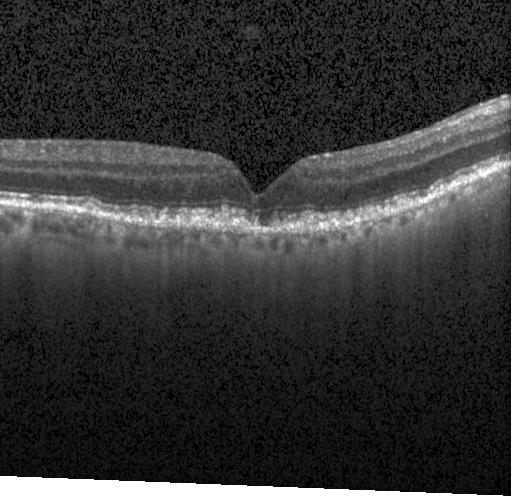

OCT B-scan. Heidelberg Spectralis OCT system — Dx: drusen.